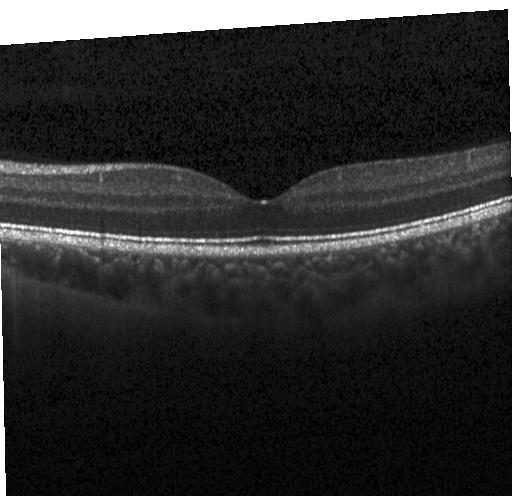 OCT B-scan. SD-OCT. Heidelberg Spectralis.
Impression: neither choroidal neovascularization, diabetic macular edema, nor drusen.